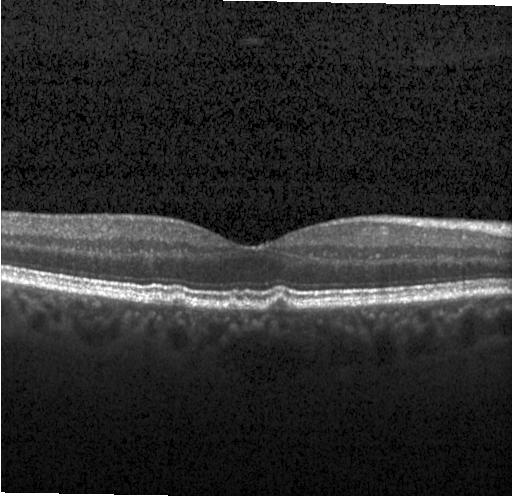

Spectral-domain OCT B-scan: sub-RPE drusenoid deposits.